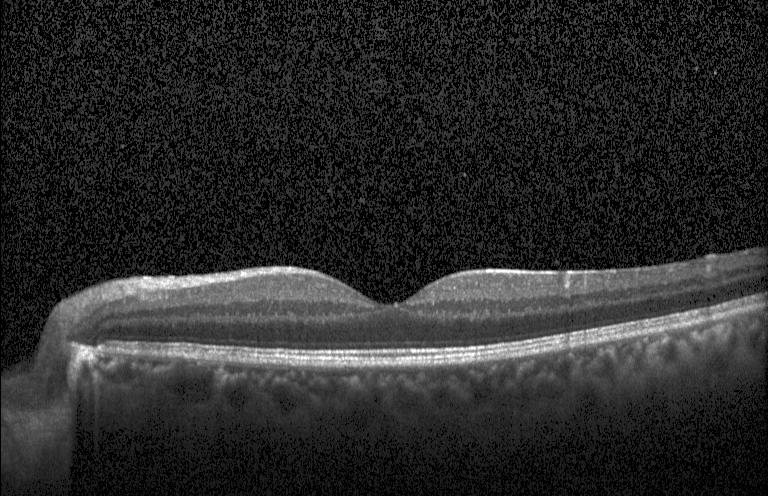
Optical coherence tomography B-scan, SD-OCT
Macular OCT: no choroidal neovascularization, diabetic macular edema, or drusen.